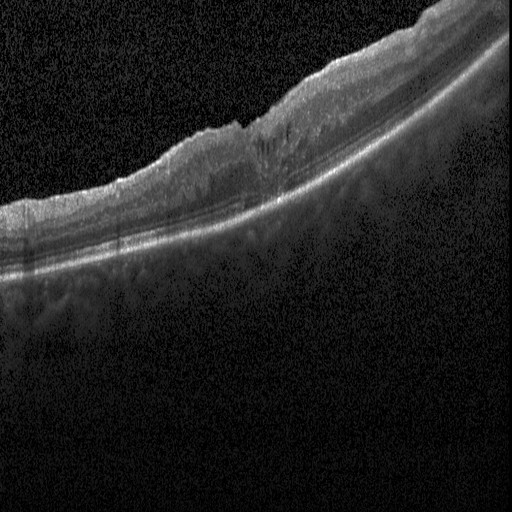
Impression: diabetic macular edema (DME).